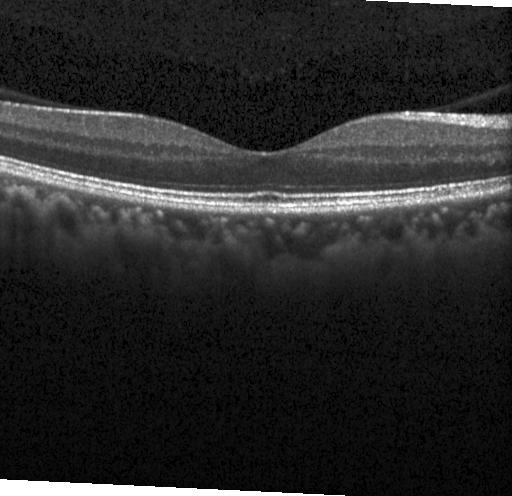
OCT B-scan showing no choroidal neovascularization, diabetic macular edema, or drusen.